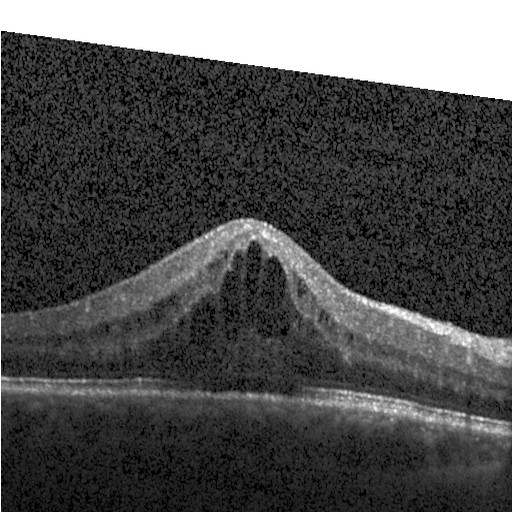

Retinal OCT B-scan. SD-OCT. Heidelberg Spectralis. This B-scan demonstrates DME.